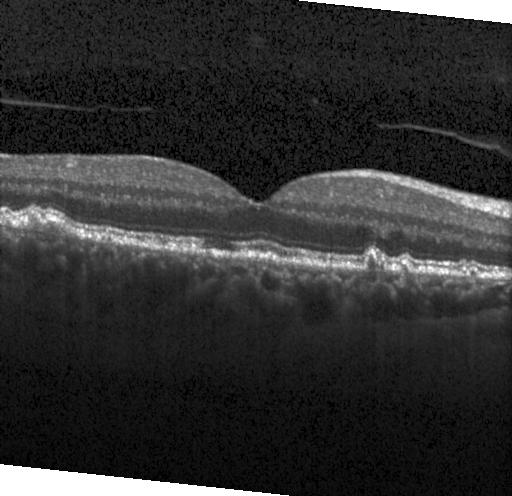

Instrument: Heidelberg Spectralis; OCT line scan.
Impression: drusen.